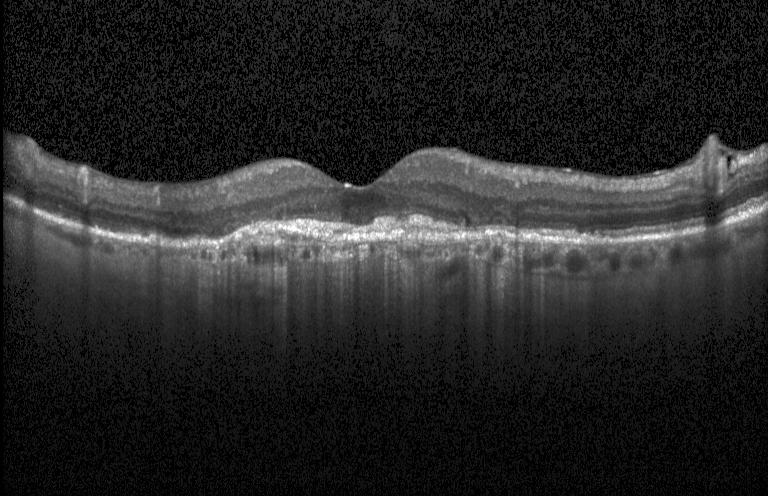
OCT B-scan. Heidelberg Spectralis OCT system. Macular scan.
Dx: choroidal neovascularization.